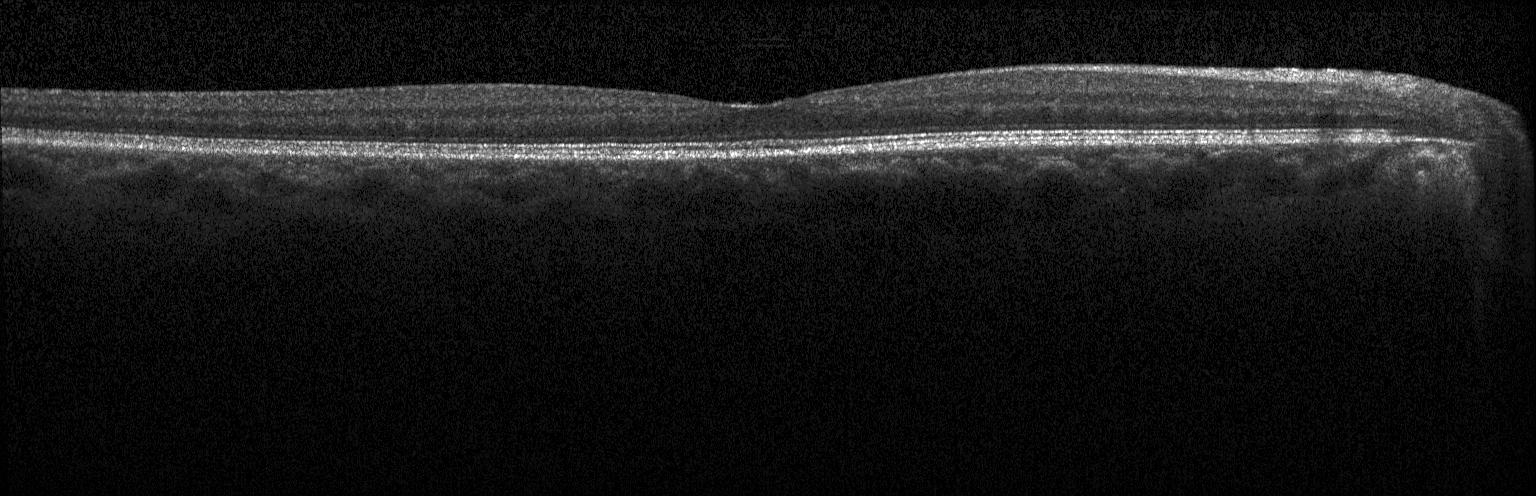
Through the macula · Heidelberg Spectralis OCT system · SD-OCT · optical coherence tomography B-scan. Diagnosis: no choroidal neovascularization, diabetic macular edema, or drusen.